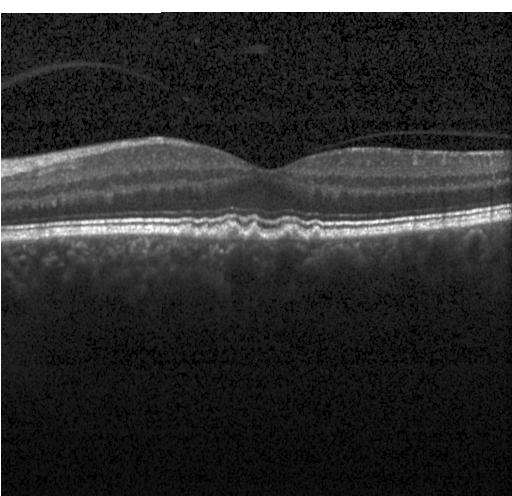

Macular scan · spectral-domain OCT · Heidelberg Spectralis · OCT line scan
Assessment: sub-RPE drusenoid deposits.